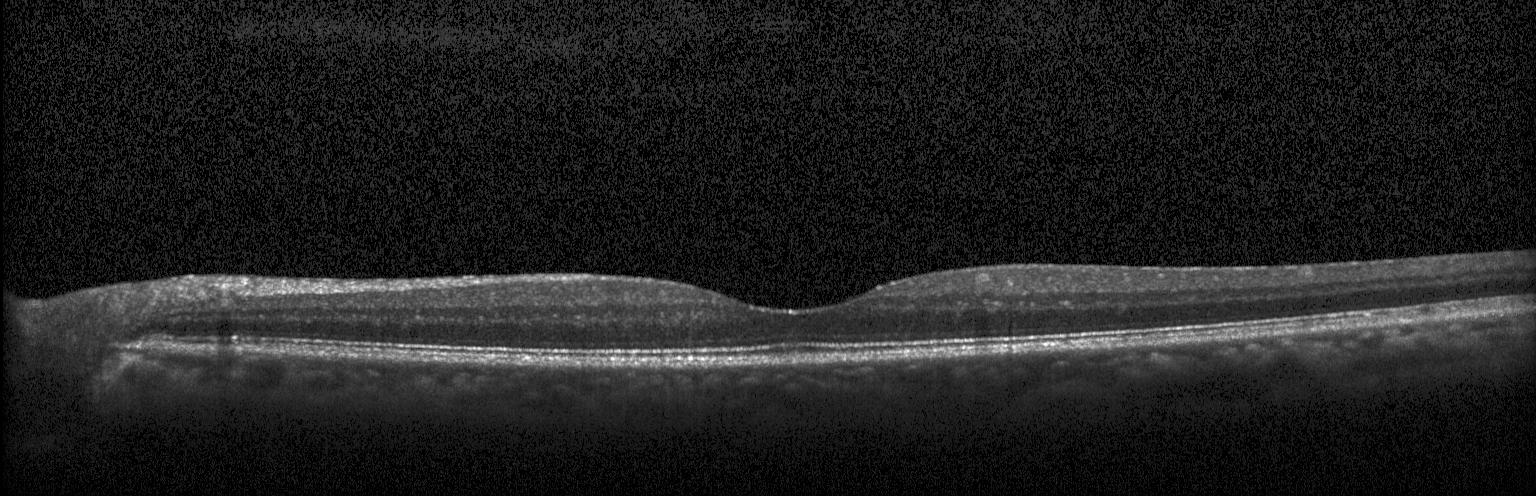
Macular scan. Retinal OCT cross-section. Heidelberg Spectralis — Finding: no choroidal neovascularization, diabetic macular edema, or drusen.